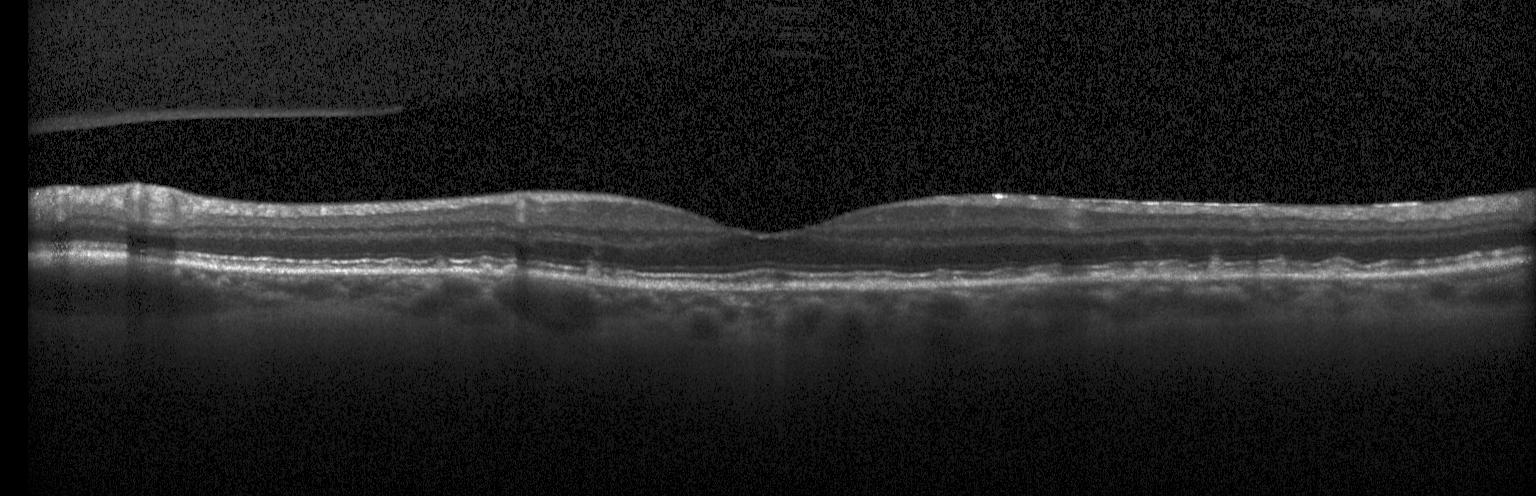

OCT finding: drusen.